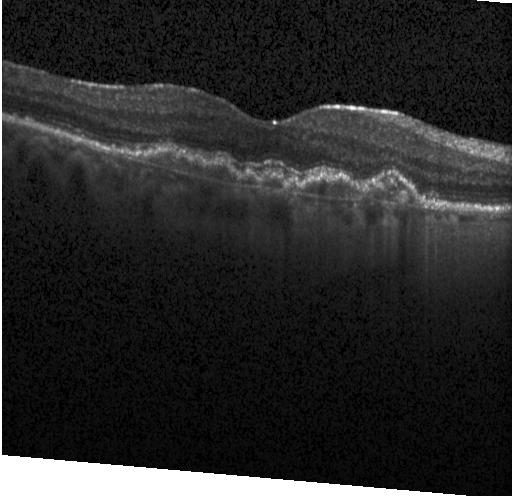
The scan shows a choroidal neovascular membrane.